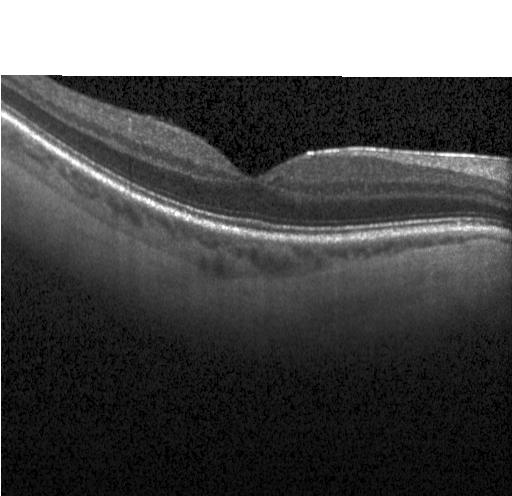
Through the macula. Optical coherence tomography B-scan. Spectral-domain optical coherence tomography. Macular OCT: no choroidal neovascularization, no diabetic macular edema, and no drusen.